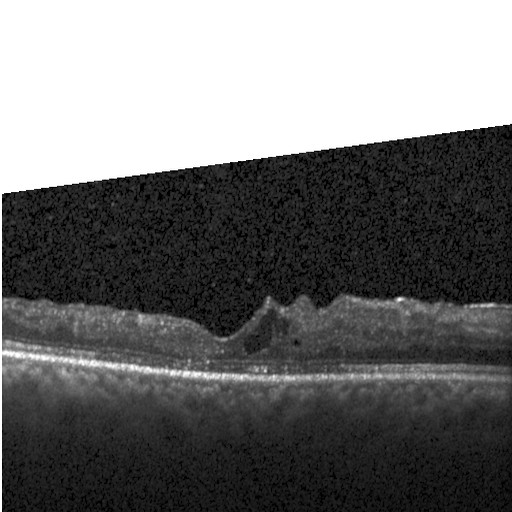
Assessment: diabetic macular edema.